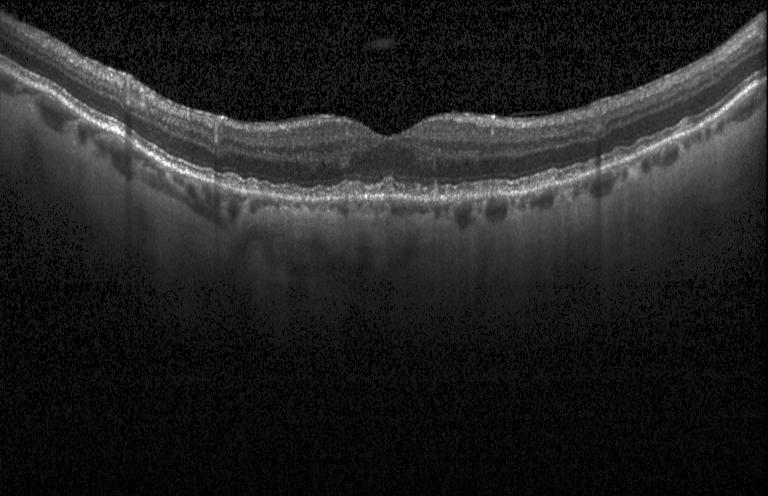
Retinal OCT cross-section showing multiple drusen.